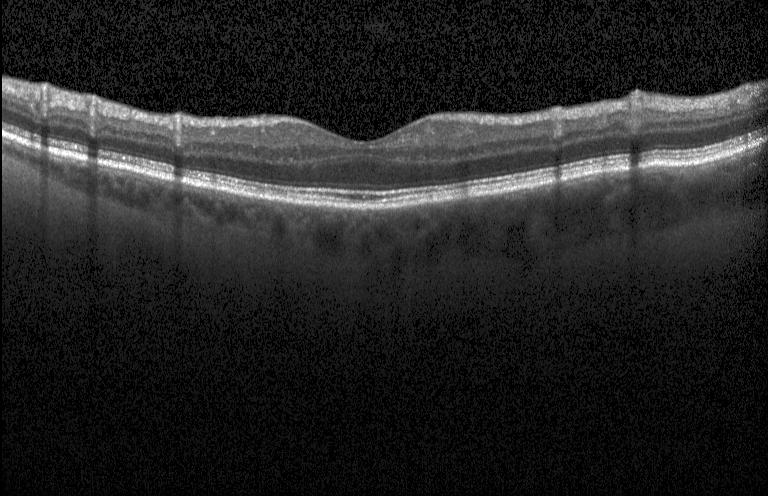

Impression: no choroidal neovascularization, no diabetic macular edema, and no drusen.